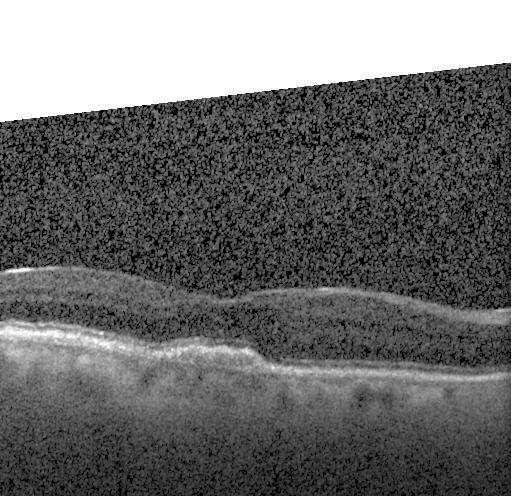

Fovea-centered; spectral-domain OCT; optical coherence tomography B-scan; acquired on a Heidelberg Spectralis.
Finding: choroidal neovascularization.